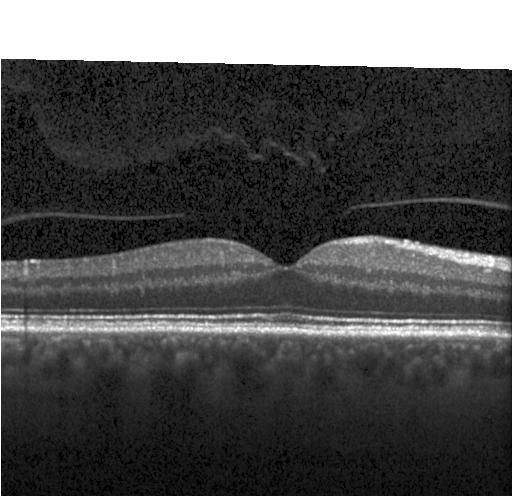 Retinal OCT B-scan. Dx: no evidence of choroidal neovascularization, diabetic macular edema, or drusen.